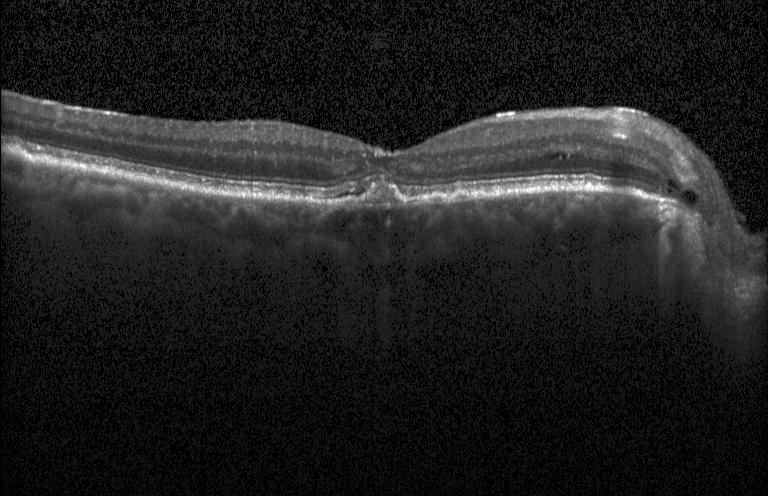
Dx: a choroidal neovascular membrane.